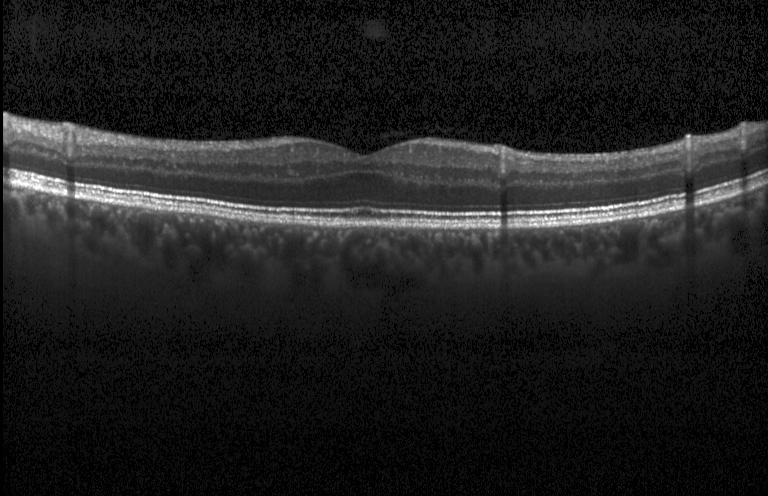
Finding: no CNV, DME, or drusen.